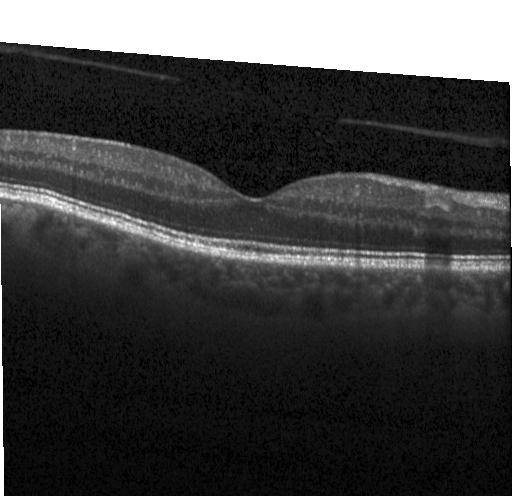

Fovea-centered · retinal OCT cross-section.
The scan shows no CNV, no DME, and no drusen.